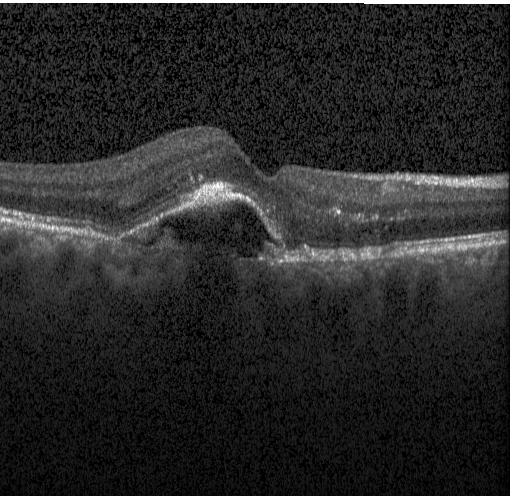

OCT line scan, spectral-domain OCT, acquired on a Heidelberg Spectralis — The scan shows a choroidal neovascular membrane.